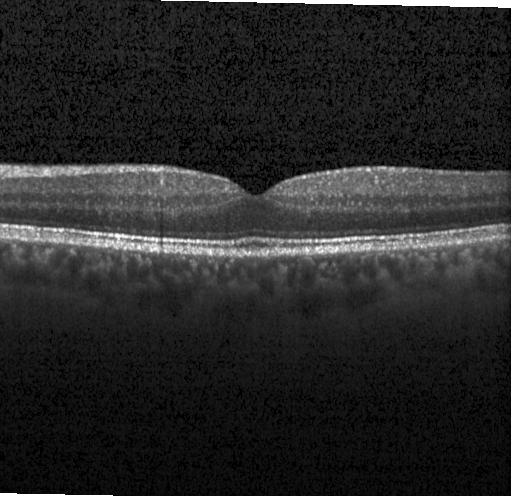 Impression: no choroidal neovascularization, diabetic macular edema, or drusen.